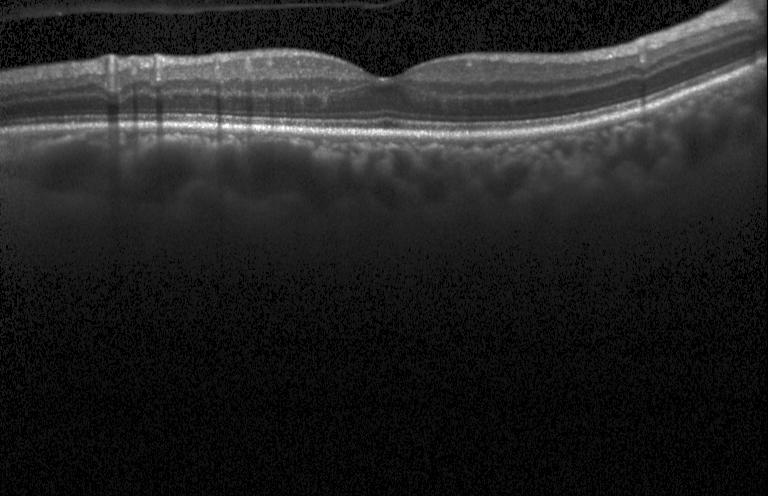 This B-scan demonstrates no CNV, no DME, and no drusen.